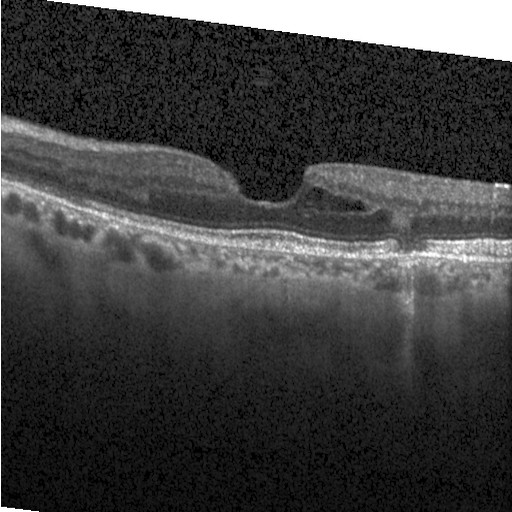

Impression: diabetic macular edema (DME).